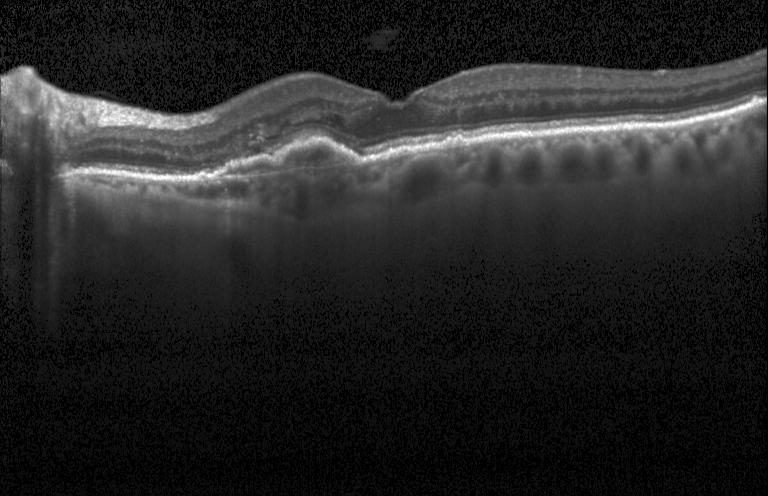 Heidelberg Spectralis OCT system; optical coherence tomography scan
Impression: choroidal neovascularization.